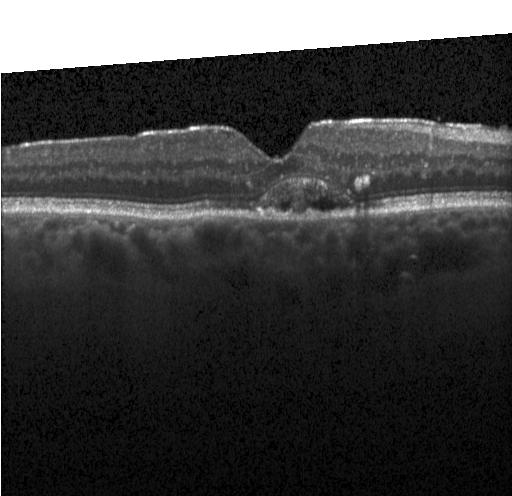
Finding: a choroidal neovascular membrane.